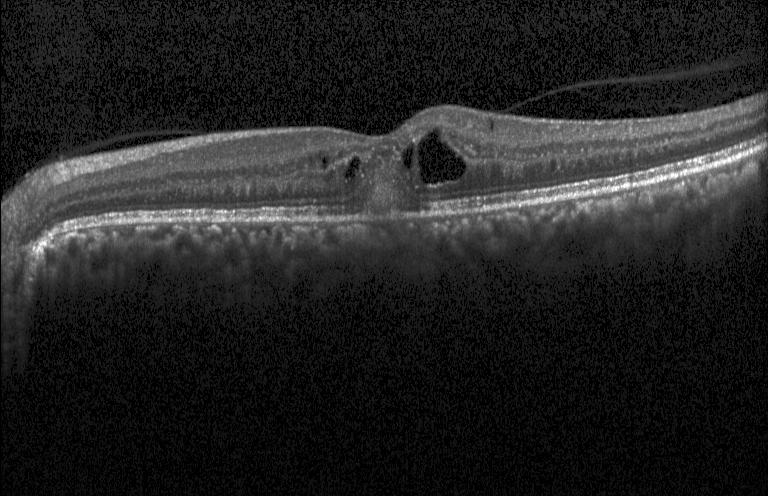 Retinal OCT B-scan, centered on the fovea, SD-OCT, acquired on a Heidelberg Spectralis. Macular OCT: a choroidal neovascular membrane.